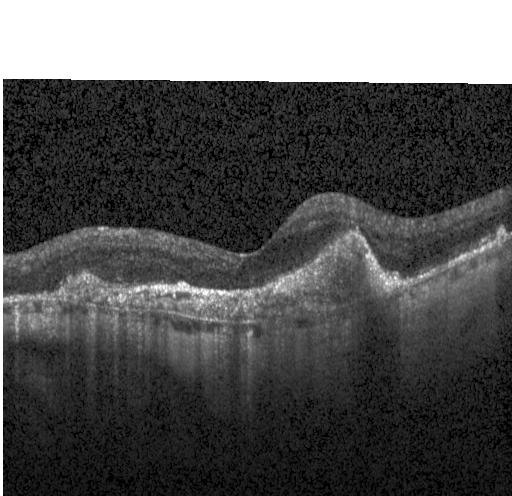
Retinal OCT cross-section
The scan shows CNV.